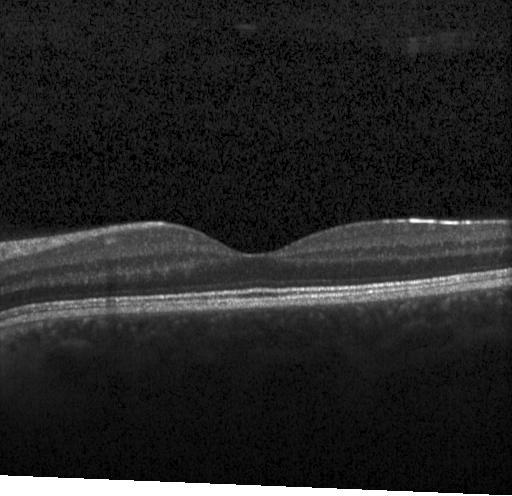
Assessment: neither CNV, DME, nor drusen.